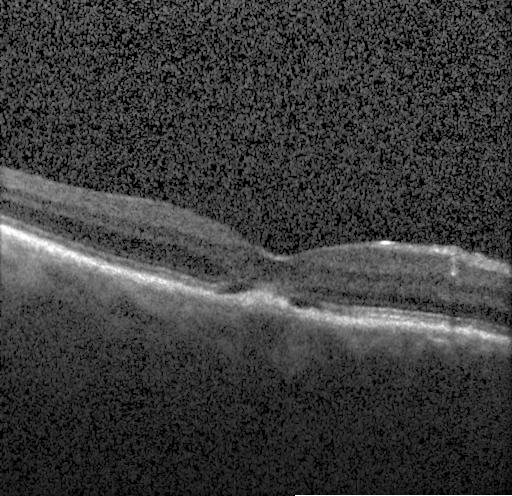

Acquired on a Heidelberg Spectralis. Spectral-domain optical coherence tomography. Macular scan. OCT line scan.
The scan shows a choroidal neovascular membrane.